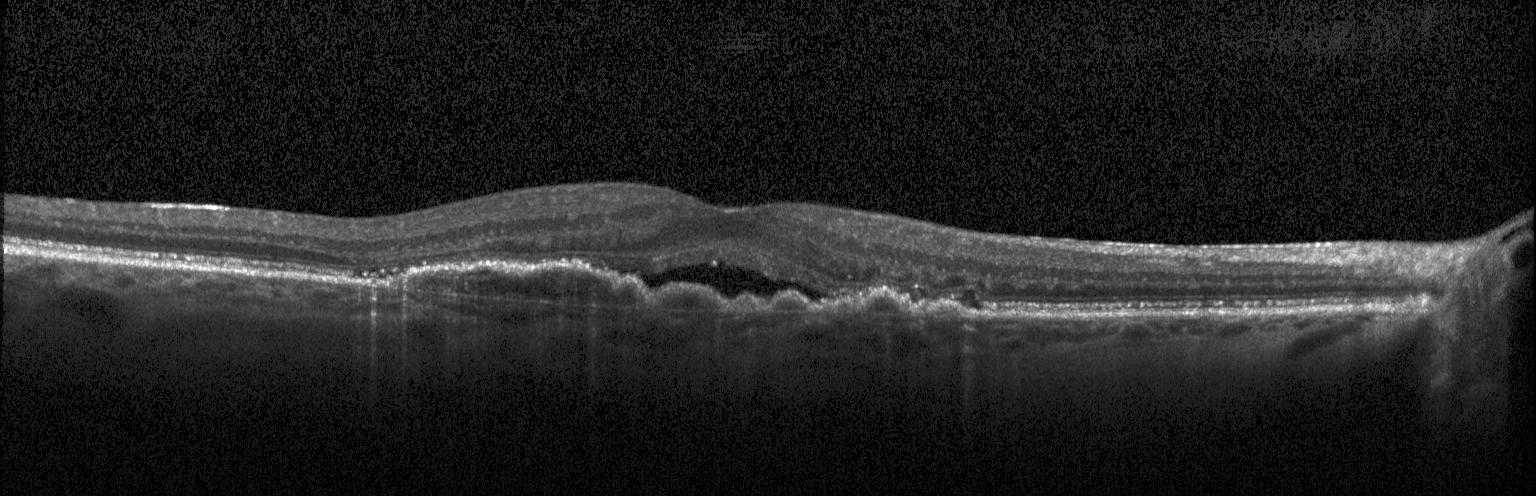
Retinal OCT cross-section.
Diagnosis: a choroidal neovascular membrane.